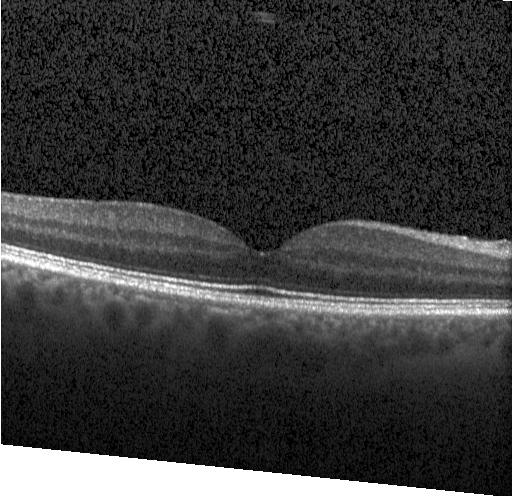
Assessment: no evidence of choroidal neovascularization, diabetic macular edema, or drusen.